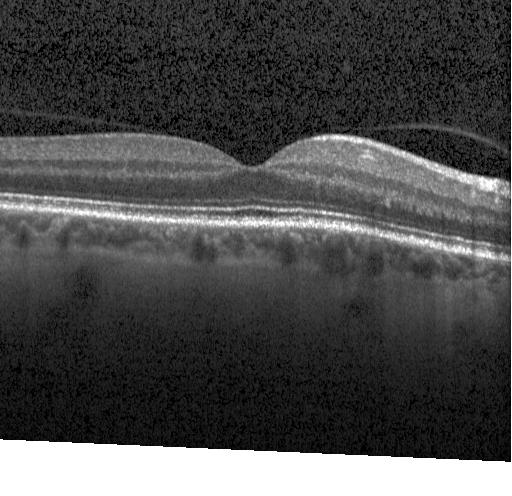 Spectral-domain OCT · optical coherence tomography scan · through the macula.
This B-scan demonstrates no choroidal neovascularization, no diabetic macular edema, and no drusen.